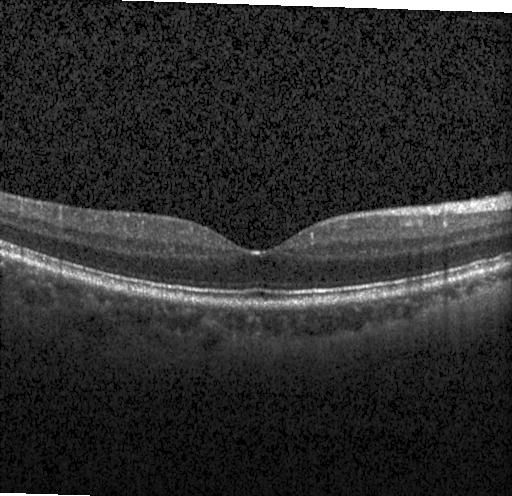

OCT B-scan · spectral-domain optical coherence tomography
This B-scan demonstrates no choroidal neovascularization, no diabetic macular edema, and no drusen.